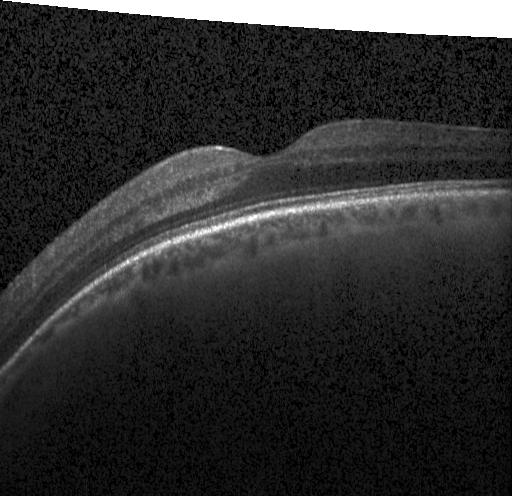 Retinal OCT B-scan; Heidelberg Spectralis OCT system; SD-OCT
Assessment: neither CNV, DME, nor drusen.